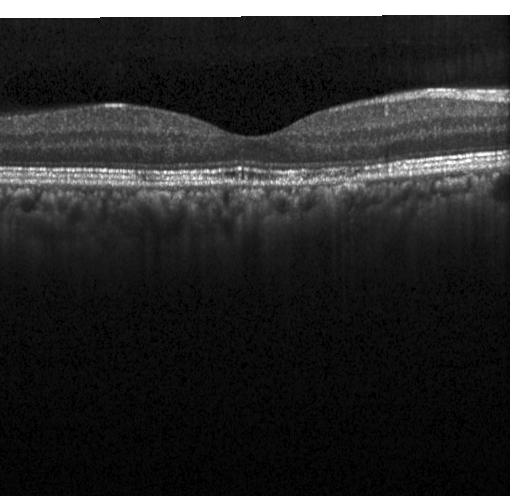 Impression: no choroidal neovascularization, diabetic macular edema, or drusen.